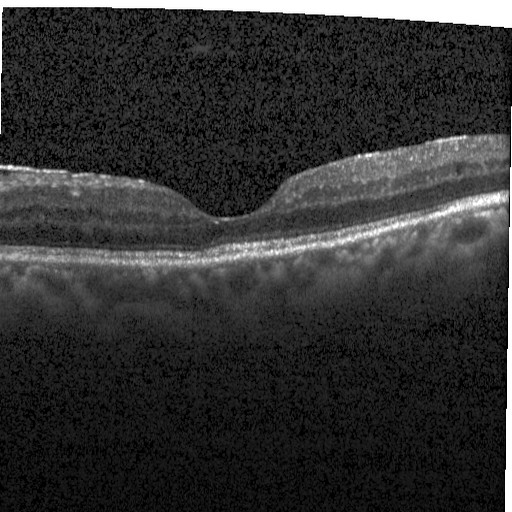

Spectral-domain optical coherence tomography. Acquired on a Heidelberg Spectralis. Optical coherence tomography scan. Macular scan — OCT finding: diabetic macular edema (DME).